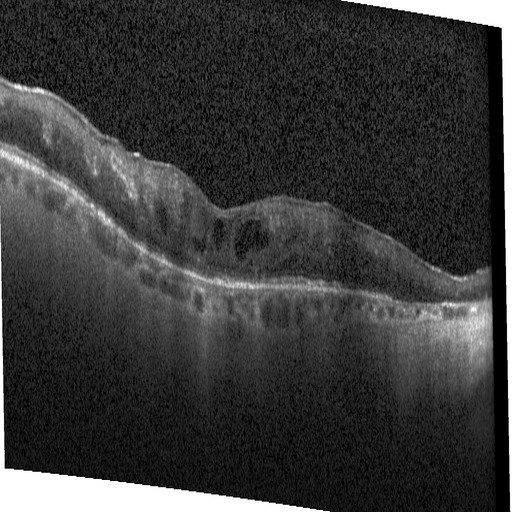
OCT B-scan showing diabetic macular edema.